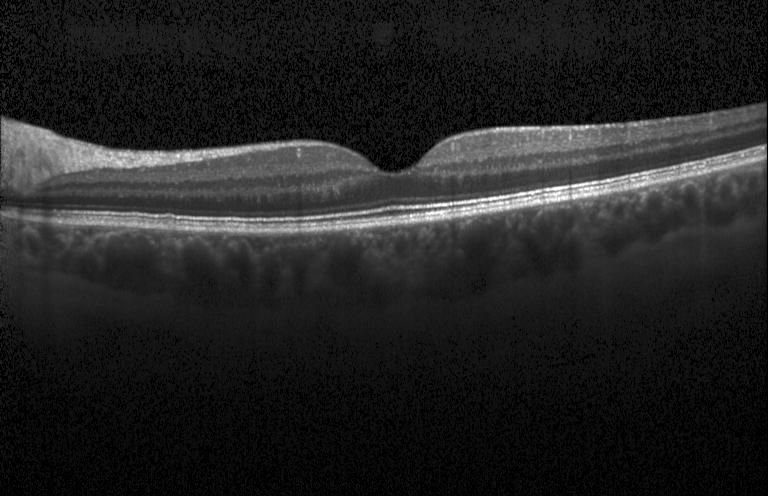
Diagnosis: no choroidal neovascularization, no diabetic macular edema, and no drusen.